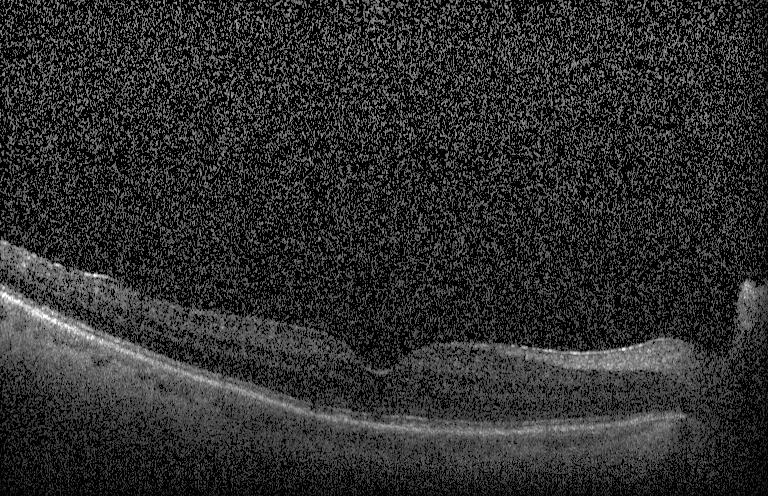
Optical coherence tomography scan.
Impression: neither CNV, DME, nor drusen.